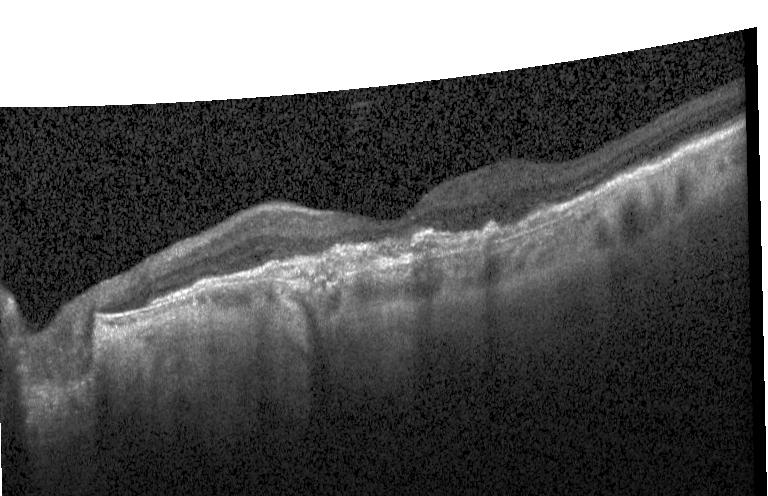 SD-OCT; optical coherence tomography scan; macular scan. CNV.